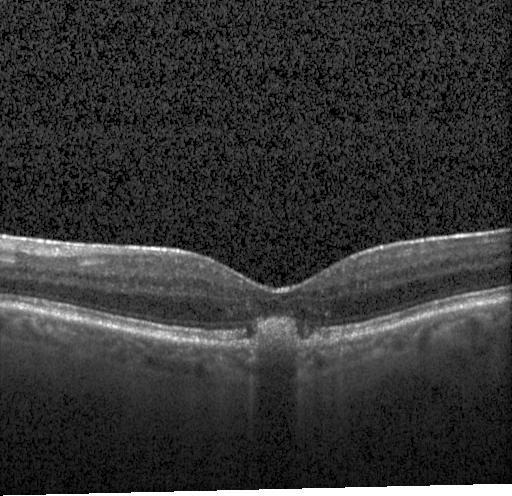 Finding: a choroidal neovascular membrane.